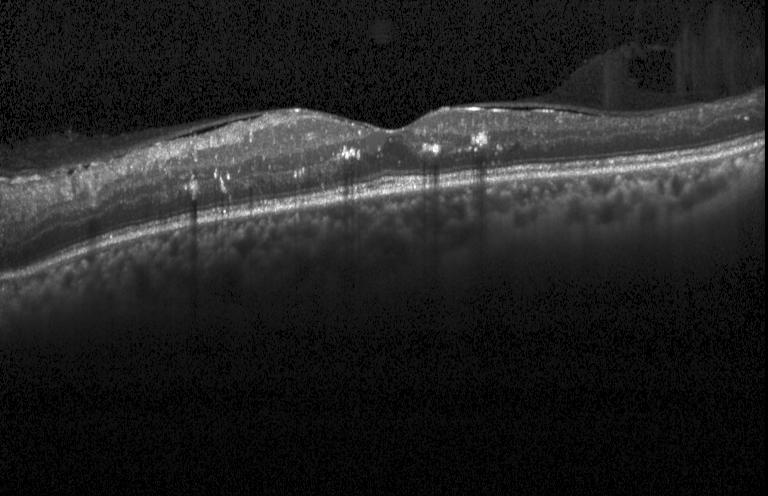
Finding: DME.